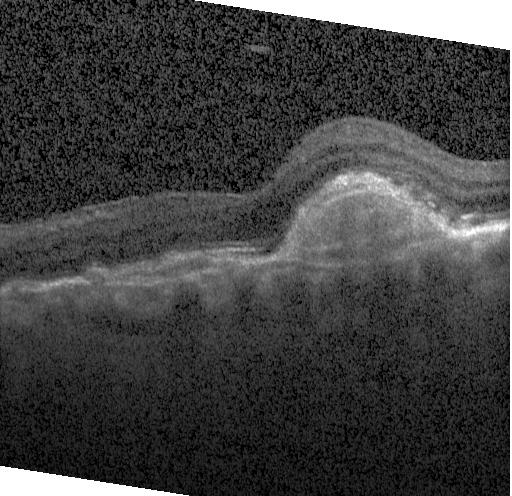 OCT line scan — Impression: a choroidal neovascular membrane.